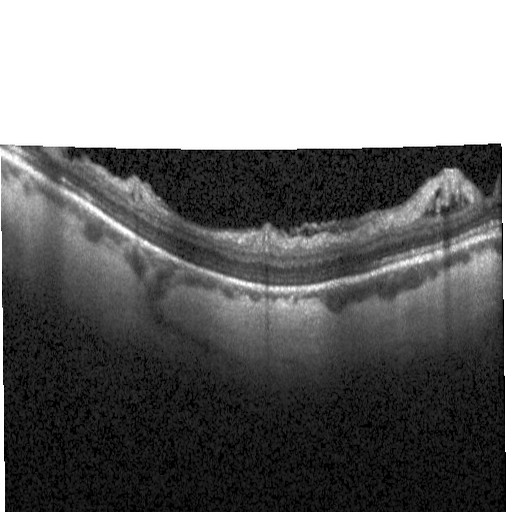

Retinal OCT cross-section — Finding: diabetic macular edema.